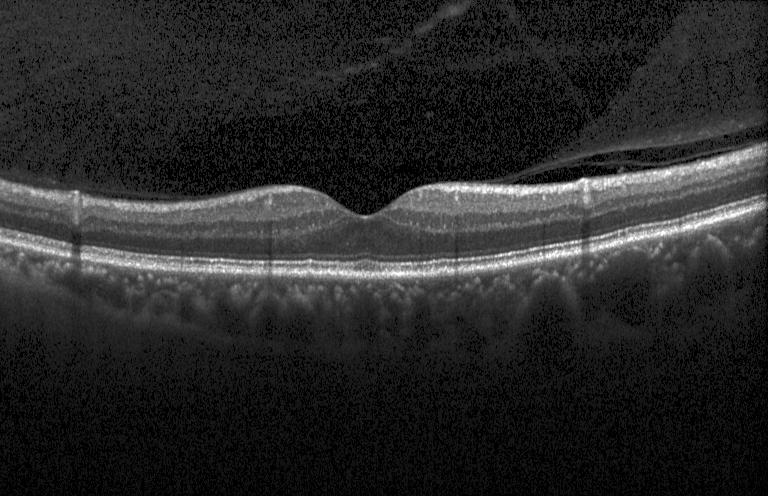 OCT finding: no evidence of CNV, DME, or drusen.